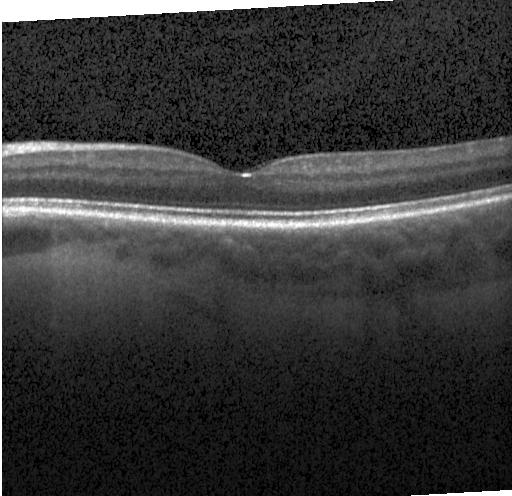

Impression: no choroidal neovascularization, diabetic macular edema, or drusen.